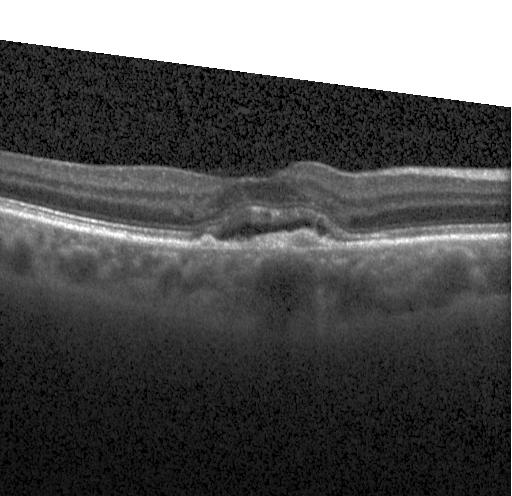 OCT B-scan showing choroidal neovascularization.